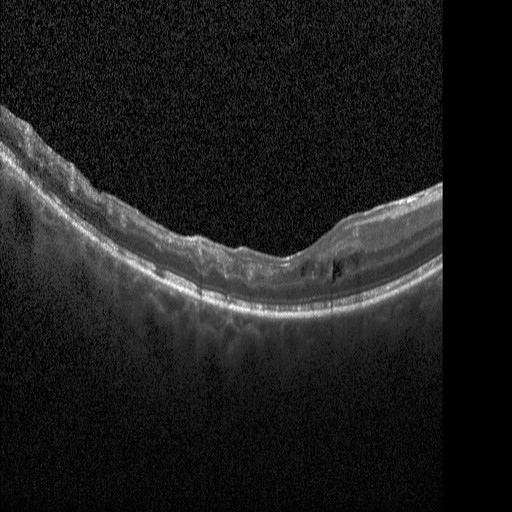
OCT line scan.
The scan shows diabetic macular edema.